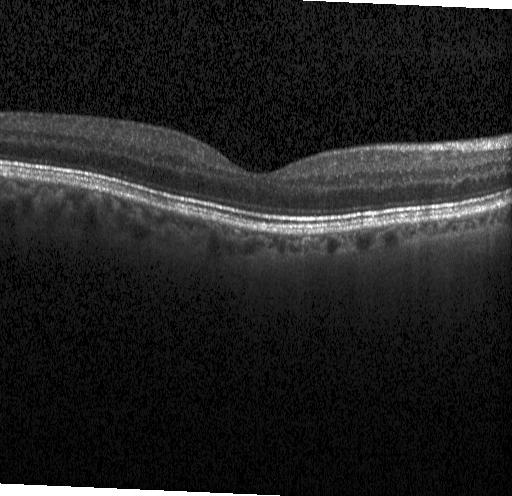 Acquired on a Heidelberg Spectralis. Fovea-centered. OCT B-scan. Dx: no choroidal neovascularization, no diabetic macular edema, and no drusen.